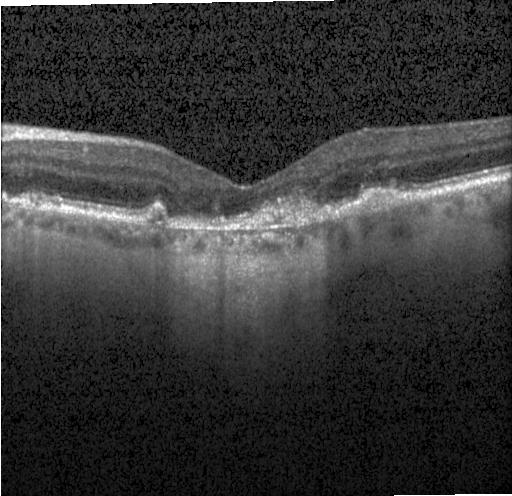

OCT B-scan; SD-OCT; fovea-centered; acquired on a Heidelberg Spectralis. OCT finding: a choroidal neovascular membrane.